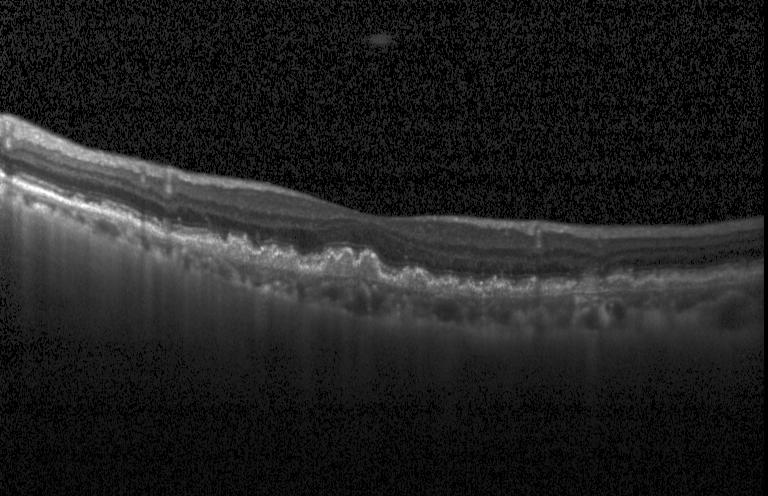

Dx: multiple drusen.